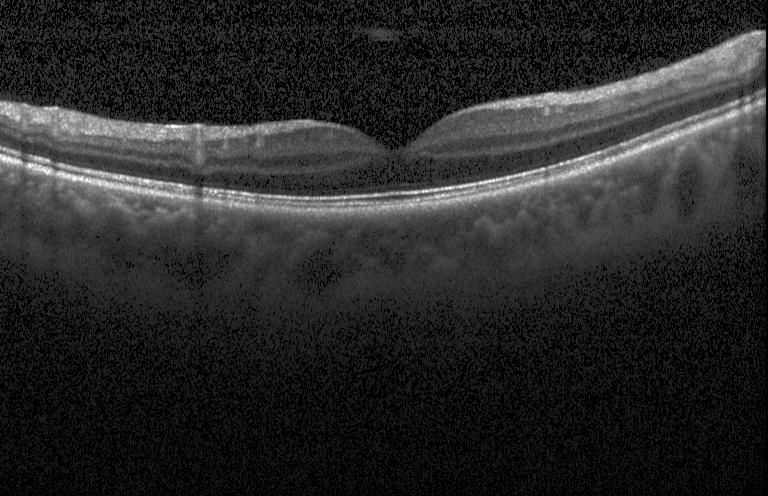
Retinal OCT B-scan. SD-OCT. Horizontal scan through the fovea.
Finding: no choroidal neovascularization, diabetic macular edema, or drusen.